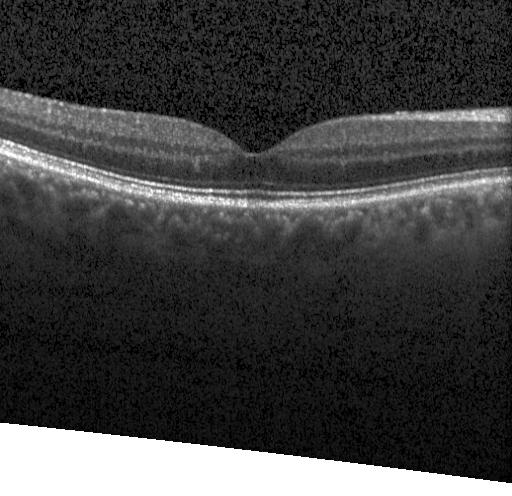
Spectral-domain optical coherence tomography; horizontal scan through the fovea; optical coherence tomography B-scan; instrument: Heidelberg Spectralis
Finding: neither choroidal neovascularization, diabetic macular edema, nor drusen.